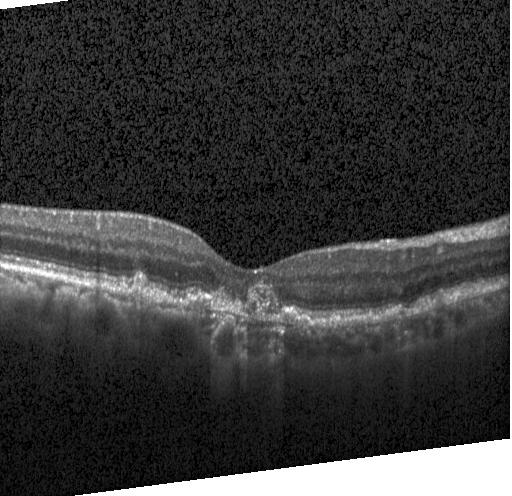

Dx: a choroidal neovascular membrane.